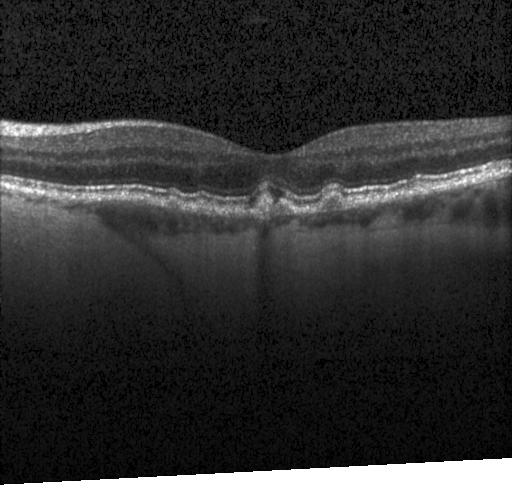 The scan shows multiple drusen.